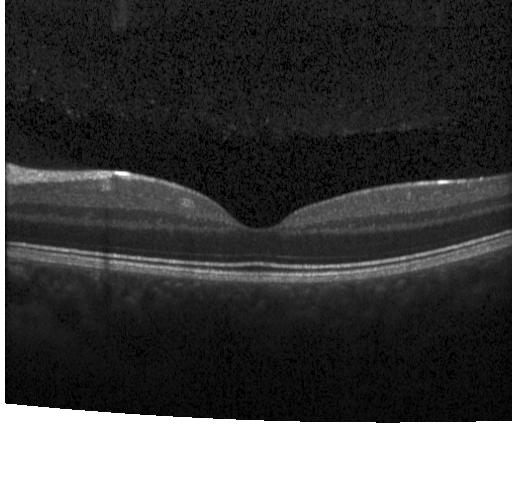

Diagnosis: no evidence of choroidal neovascularization, diabetic macular edema, or drusen.